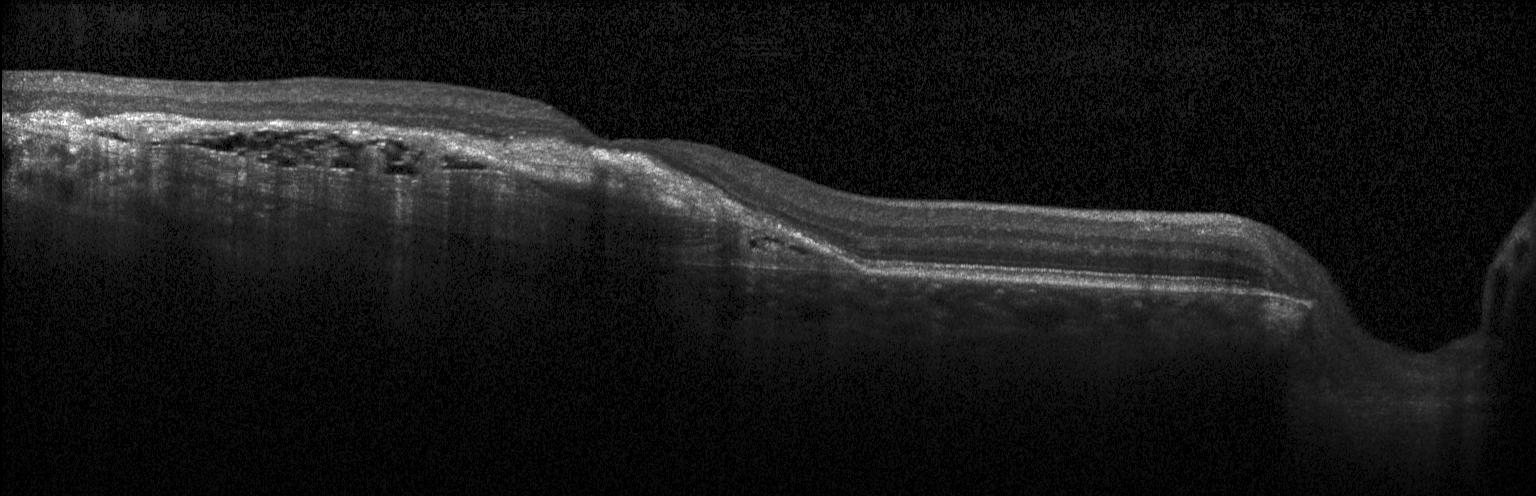

Macular OCT: a choroidal neovascular membrane.